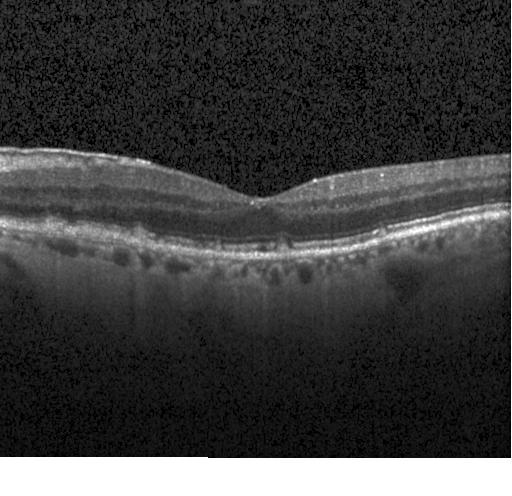
Horizontal scan through the fovea · Heidelberg Spectralis OCT system · optical coherence tomography scan — Diagnosis: drusen.